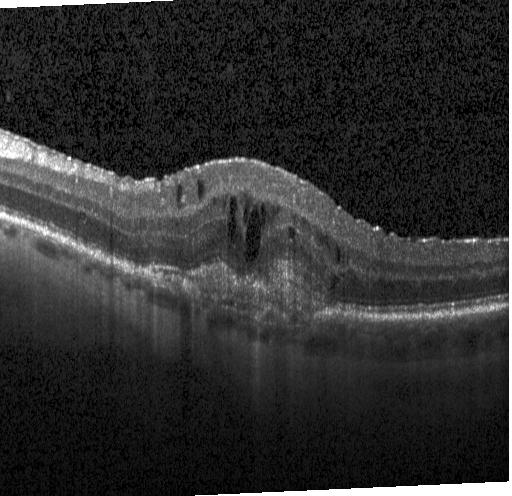 Instrument: Heidelberg Spectralis. Macular scan. Spectral-domain OCT. Optical coherence tomography scan. OCT finding: choroidal neovascularization.